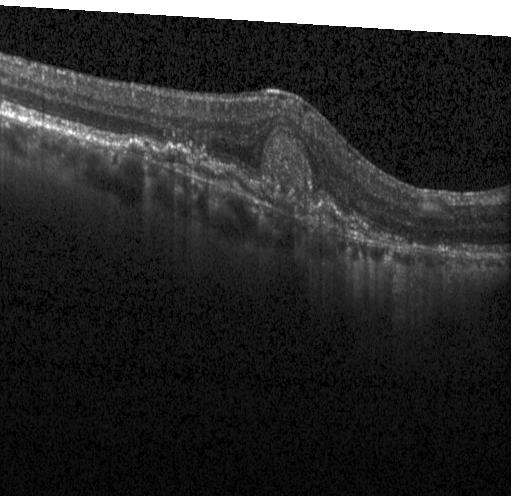 Finding: a choroidal neovascular membrane.